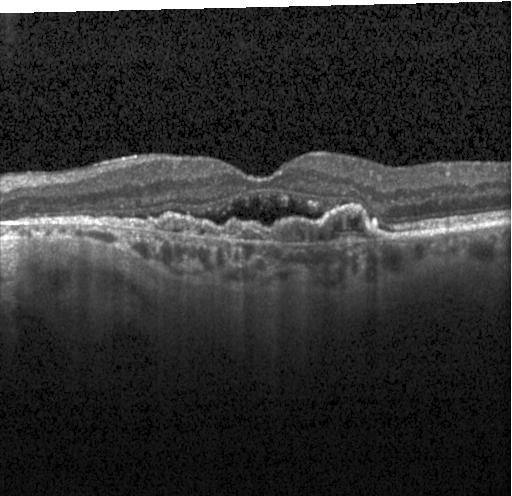 OCT line scan. Assessment: choroidal neovascularization (CNV).